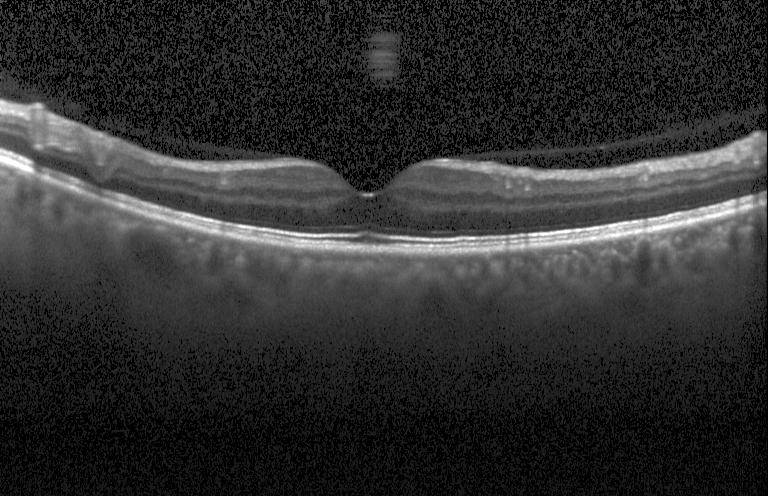

Instrument: Heidelberg Spectralis, macular scan, OCT B-scan — Dx: no CNV, no DME, and no drusen.